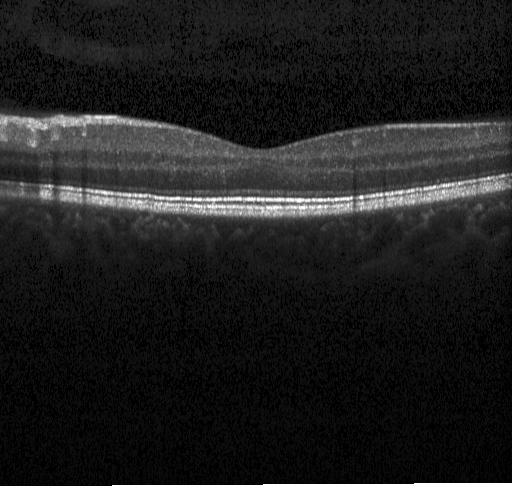 Spectral-domain OCT B-scan: no choroidal neovascularization, no diabetic macular edema, and no drusen.